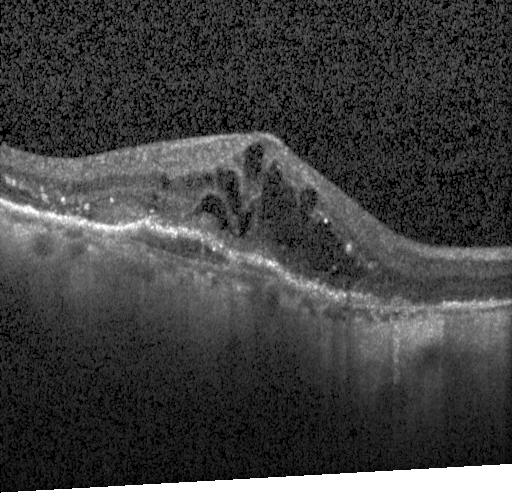
Diagnosis: CNV.